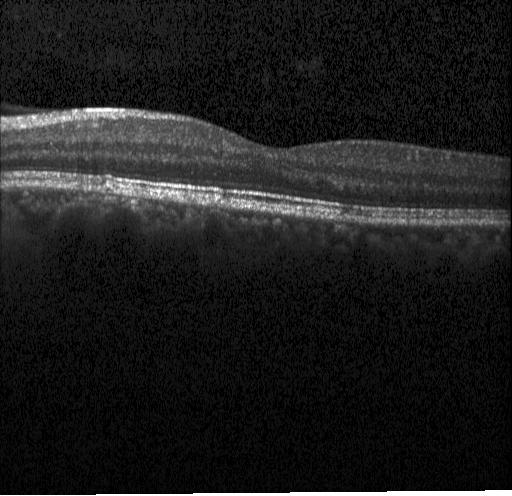

Dx: drusen.